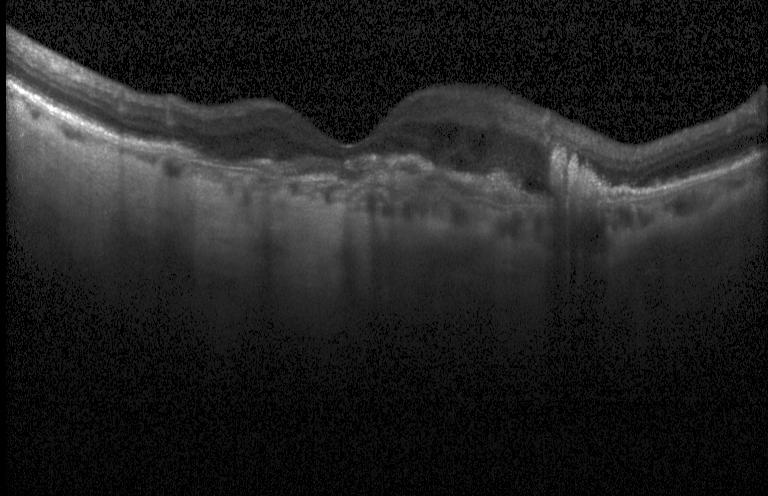
Spectral-domain OCT B-scan: choroidal neovascularization (CNV).